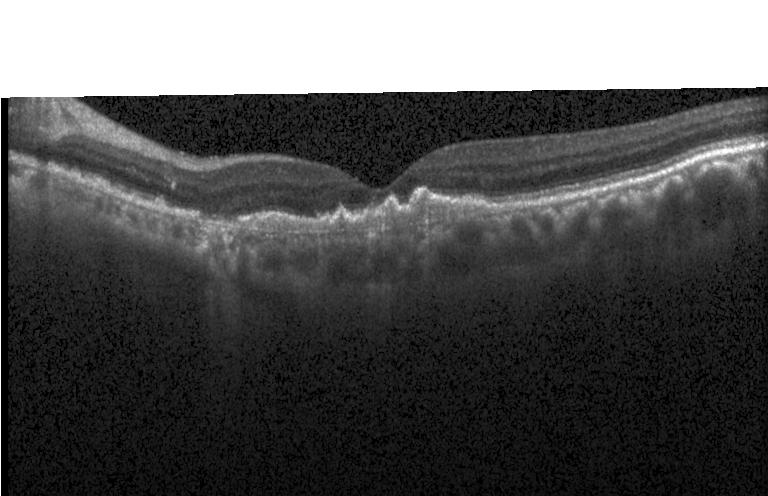 Fovea-centered. Retinal OCT cross-section. Finding: CNV.